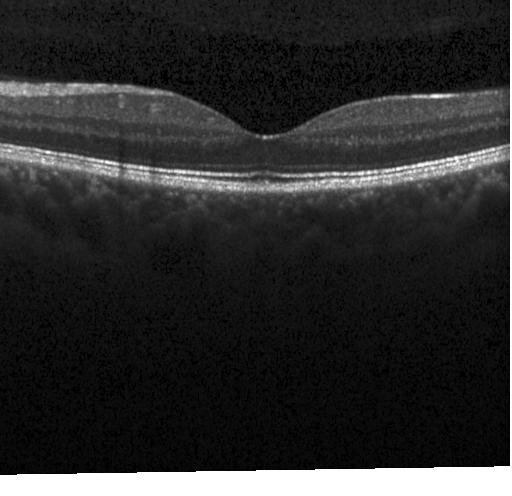

Impression: neither choroidal neovascularization, diabetic macular edema, nor drusen.